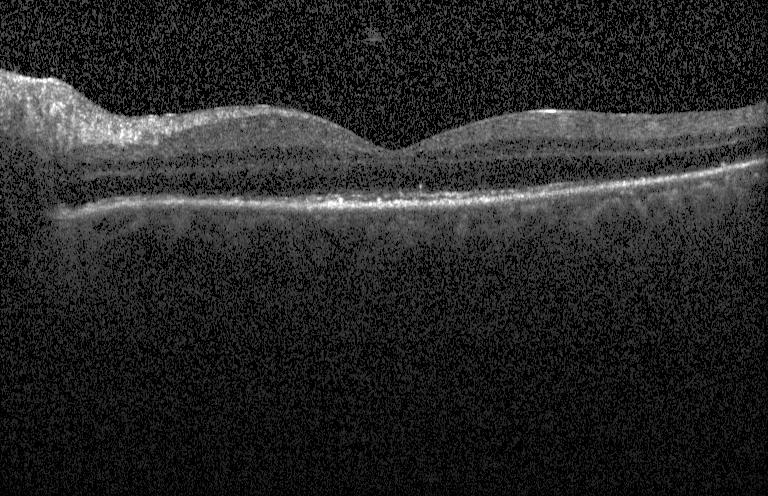 OCT B-scan
This B-scan demonstrates no choroidal neovascularization, diabetic macular edema, or drusen.